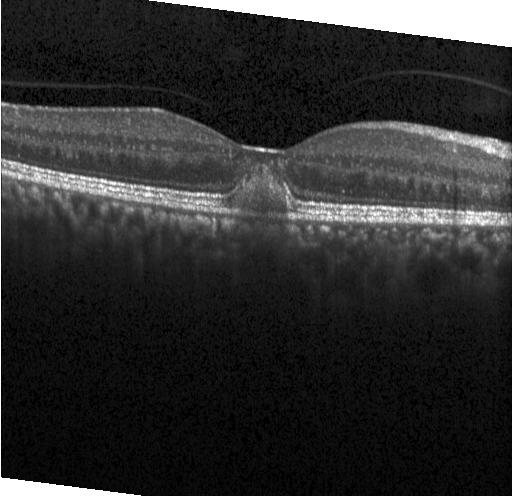
Macular scan · OCT B-scan.
Finding: a choroidal neovascular membrane.